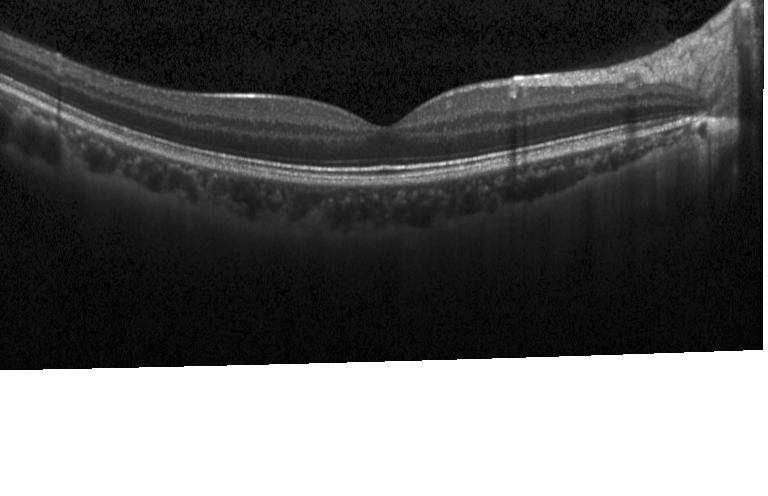

Diagnosis: neither CNV, DME, nor drusen.